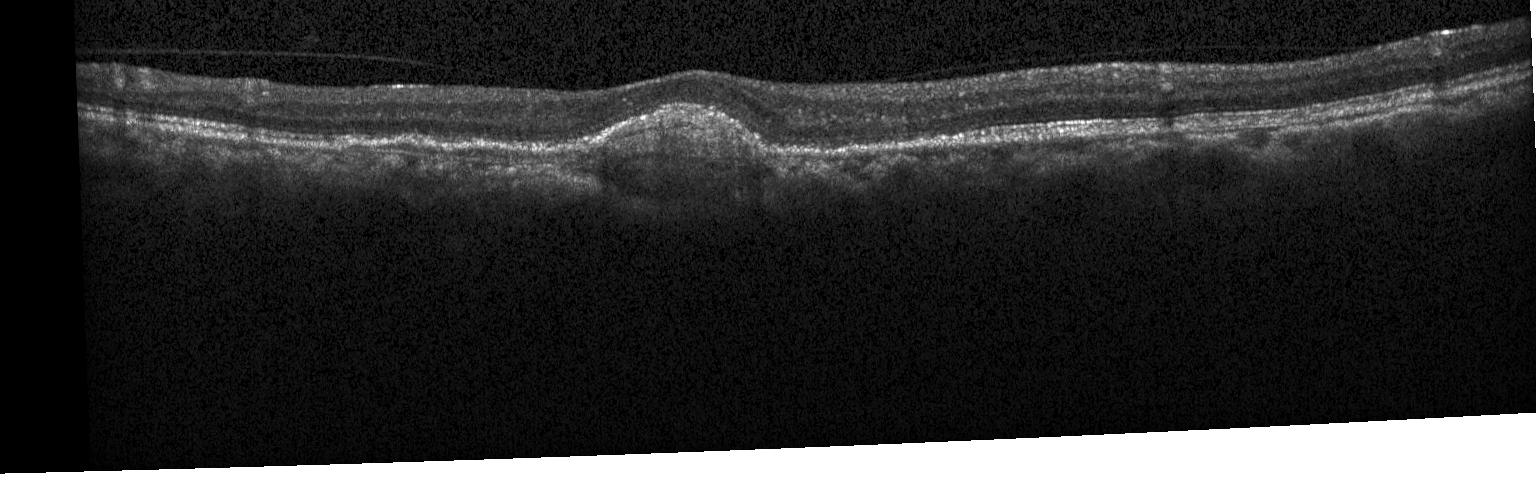

Assessment: a choroidal neovascular membrane.